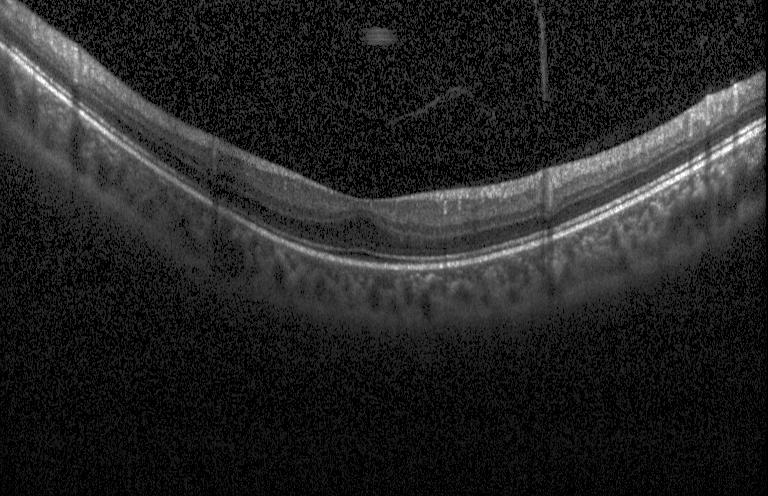 Spectral-domain OCT. Retinal OCT B-scan. Assessment: neither choroidal neovascularization, diabetic macular edema, nor drusen.